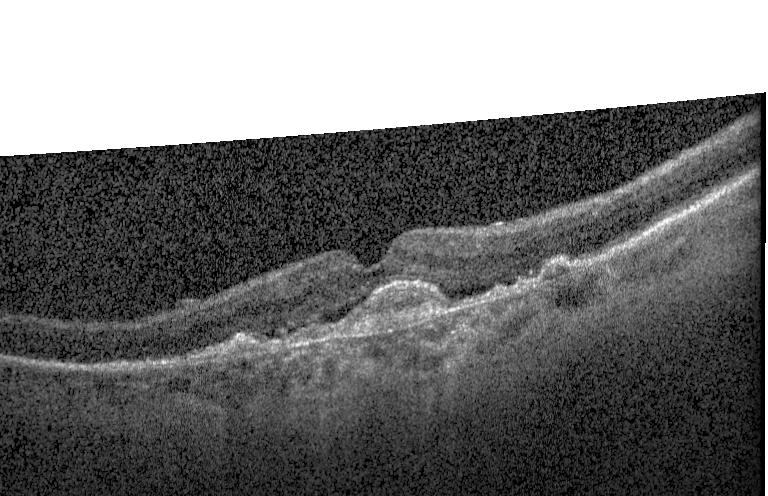 Instrument: Heidelberg Spectralis; retinal OCT B-scan; spectral-domain optical coherence tomography
The scan shows a choroidal neovascular membrane.